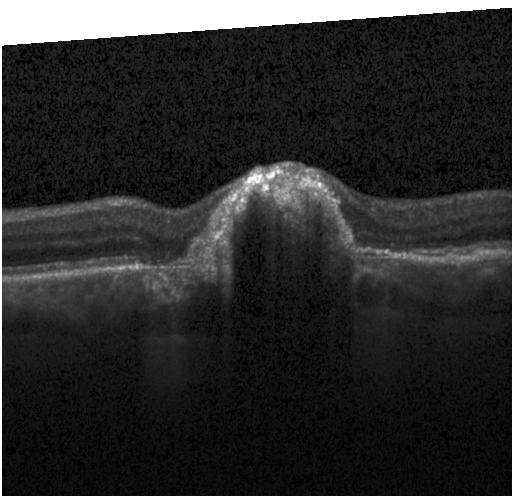
OCT finding: CNV.